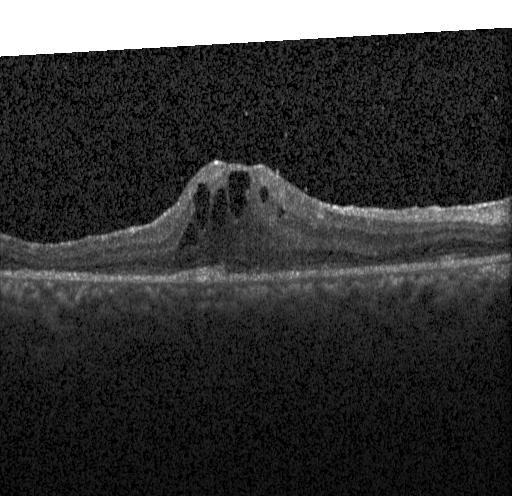 Dx: a choroidal neovascular membrane.